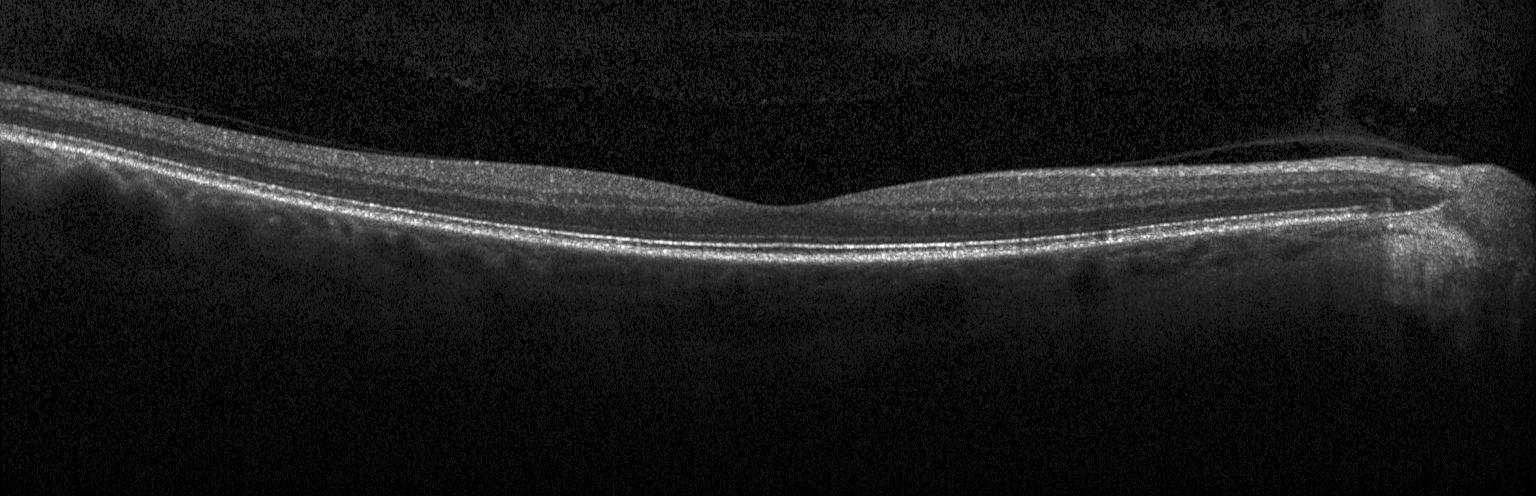
This B-scan demonstrates neither CNV, DME, nor drusen.